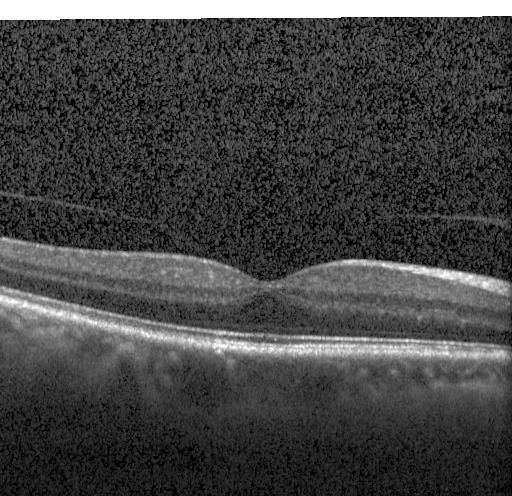

Optical coherence tomography scan; spectral-domain optical coherence tomography. No choroidal neovascularization, diabetic macular edema, or drusen.